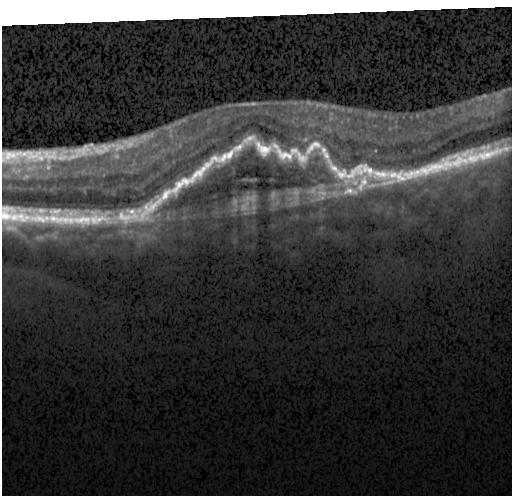 Spectral-domain optical coherence tomography · optical coherence tomography scan · horizontal scan through the fovea. The scan shows a choroidal neovascular membrane.